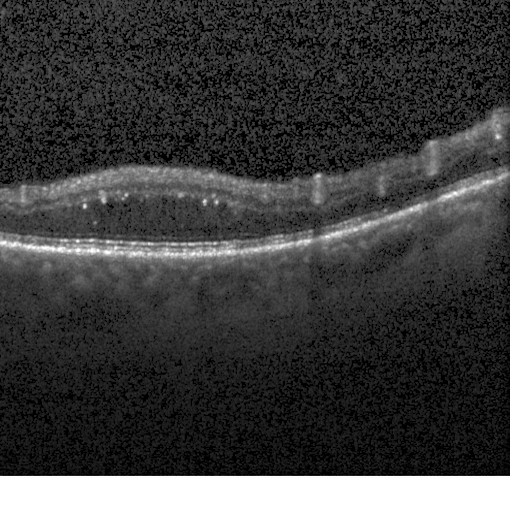 Retinal OCT B-scan
Diabetic macular edema.